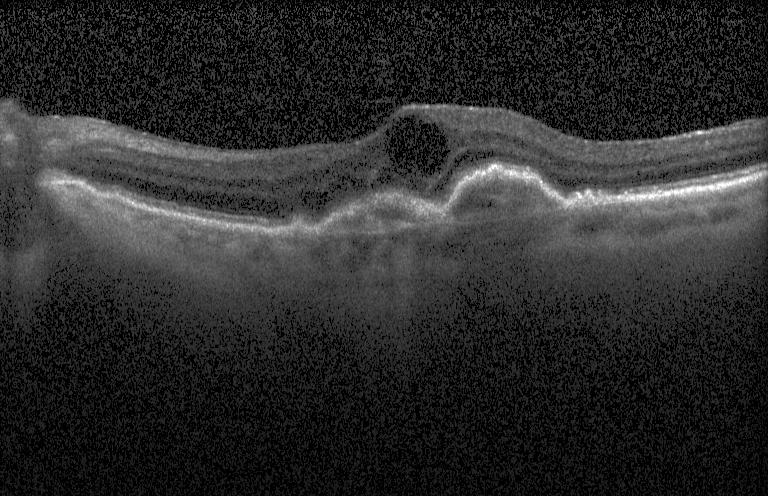

Assessment: a choroidal neovascular membrane.